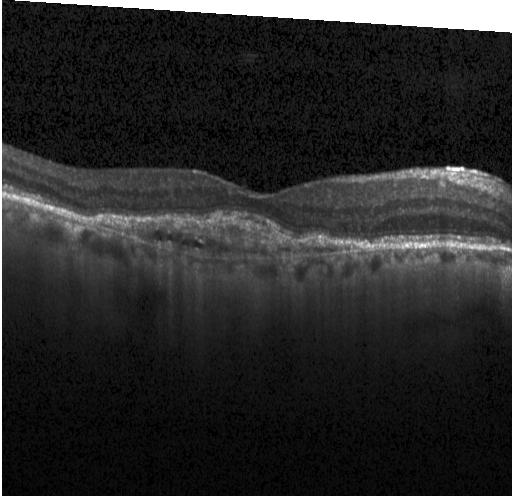

SD-OCT. Retinal OCT cross-section. Instrument: Heidelberg Spectralis. Fovea-centered — Finding: choroidal neovascularization (CNV).